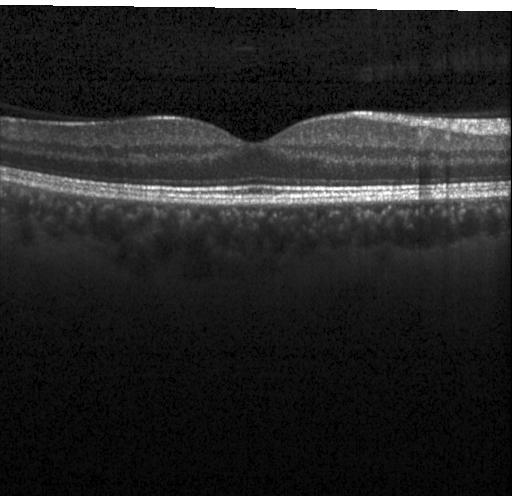

Spectral-domain optical coherence tomography. Retinal OCT B-scan. Horizontal scan through the fovea — Dx: no choroidal neovascularization, no diabetic macular edema, and no drusen.